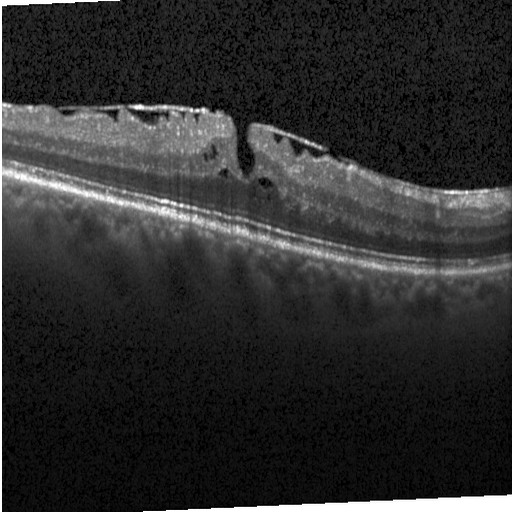

The scan shows diabetic macular edema (DME).